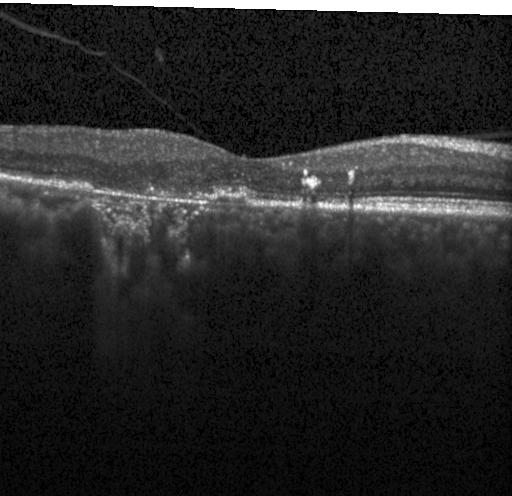

Impression: choroidal neovascularization.